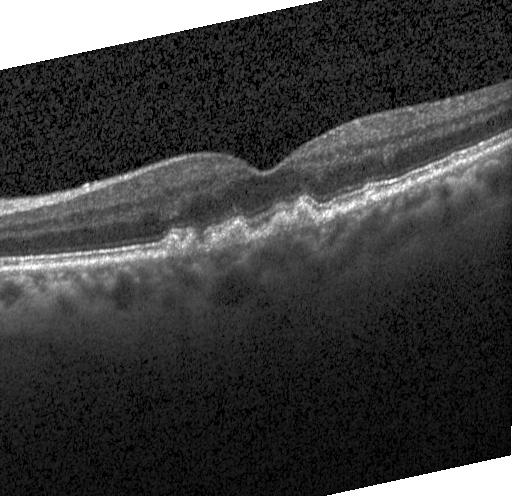
Macular scan; SD-OCT; OCT B-scan.
The scan shows drusen.